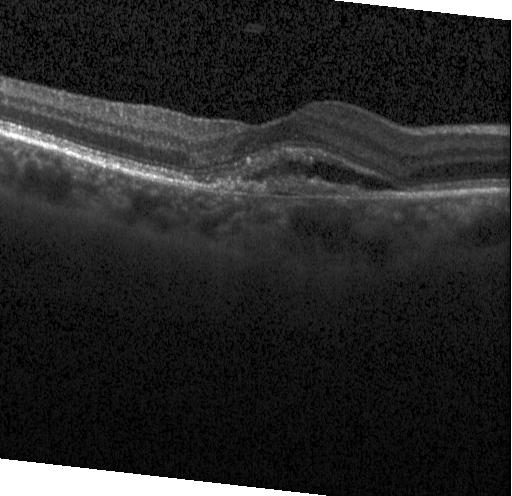 Through the macula. Instrument: Heidelberg Spectralis. Optical coherence tomography scan
Finding: a choroidal neovascular membrane.